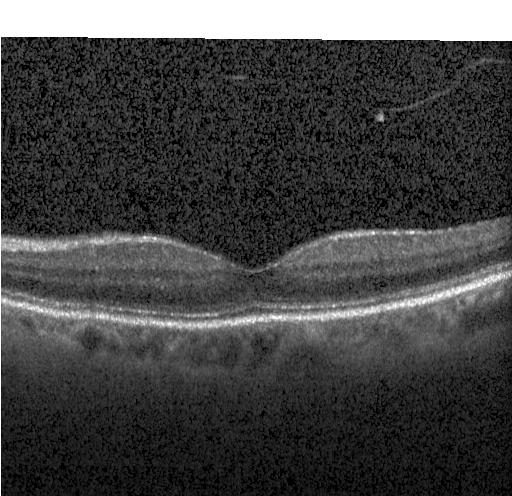

This B-scan demonstrates no choroidal neovascularization, no diabetic macular edema, and no drusen.